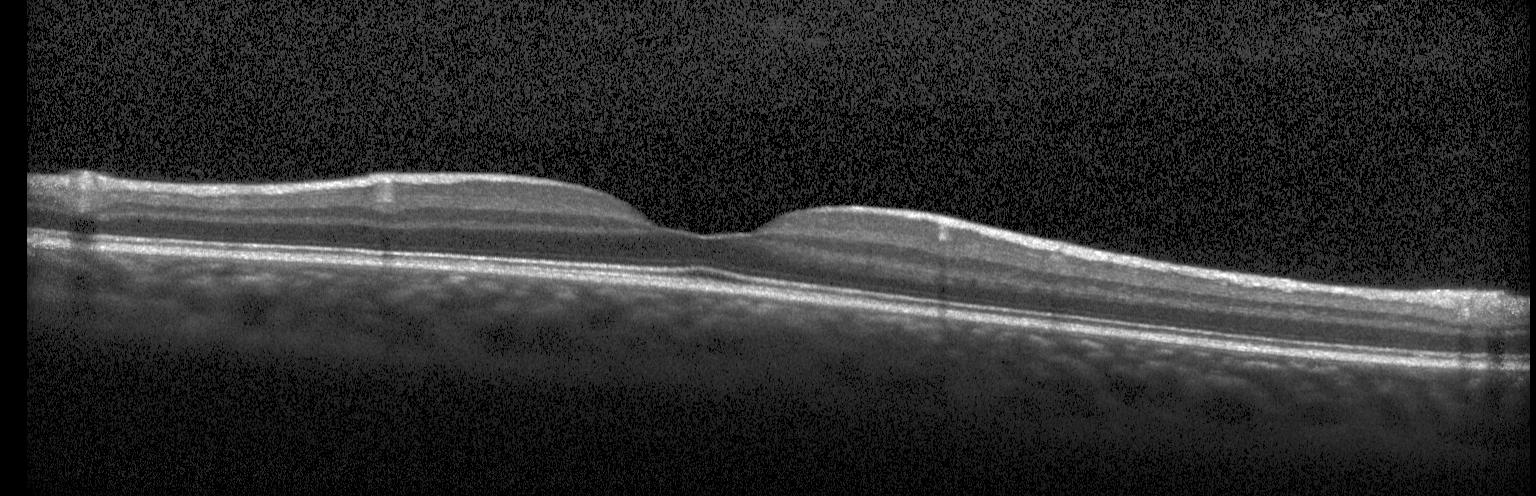 Dx: neither choroidal neovascularization, diabetic macular edema, nor drusen.